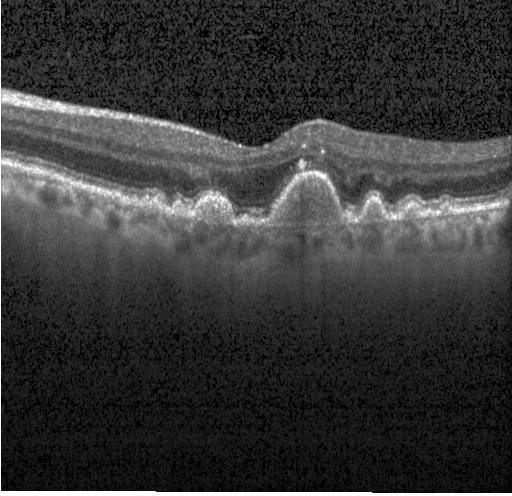

Impression: sub-RPE drusenoid deposits.